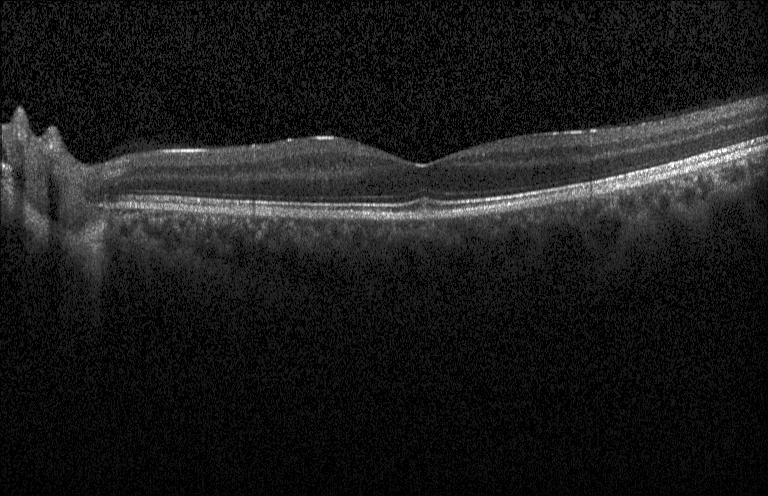

Retinal OCT B-scan
Finding: neither choroidal neovascularization, diabetic macular edema, nor drusen.